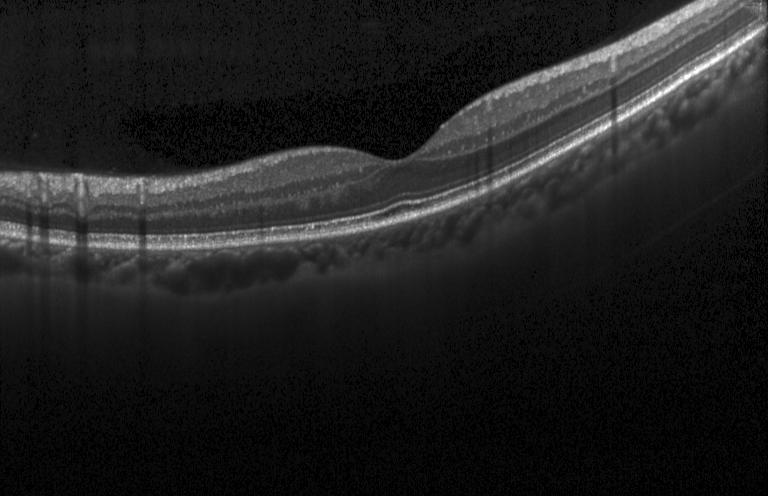
OCT B-scan, Heidelberg Spectralis OCT system, spectral-domain OCT
No evidence of choroidal neovascularization, diabetic macular edema, or drusen.